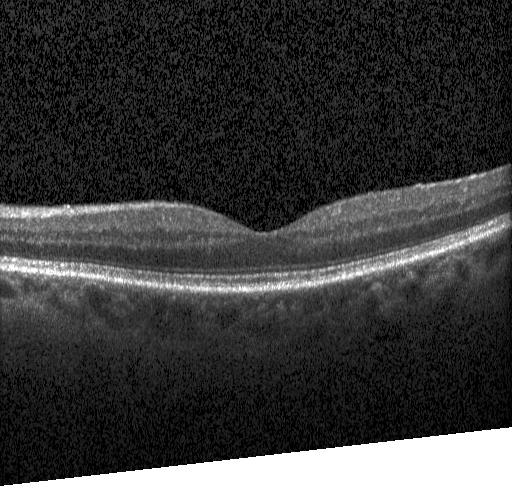 OCT B-scan showing neither choroidal neovascularization, diabetic macular edema, nor drusen.